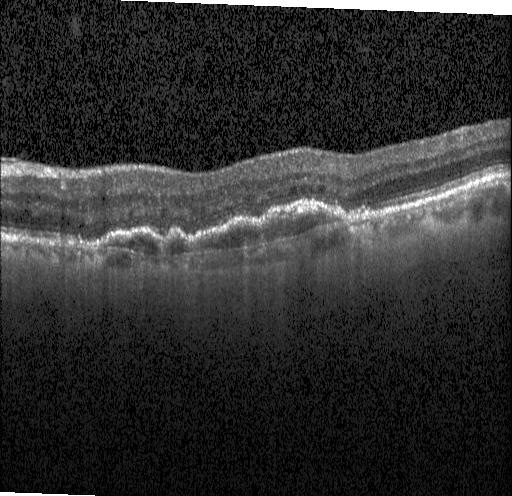

Spectral-domain OCT B-scan: choroidal neovascularization (CNV).